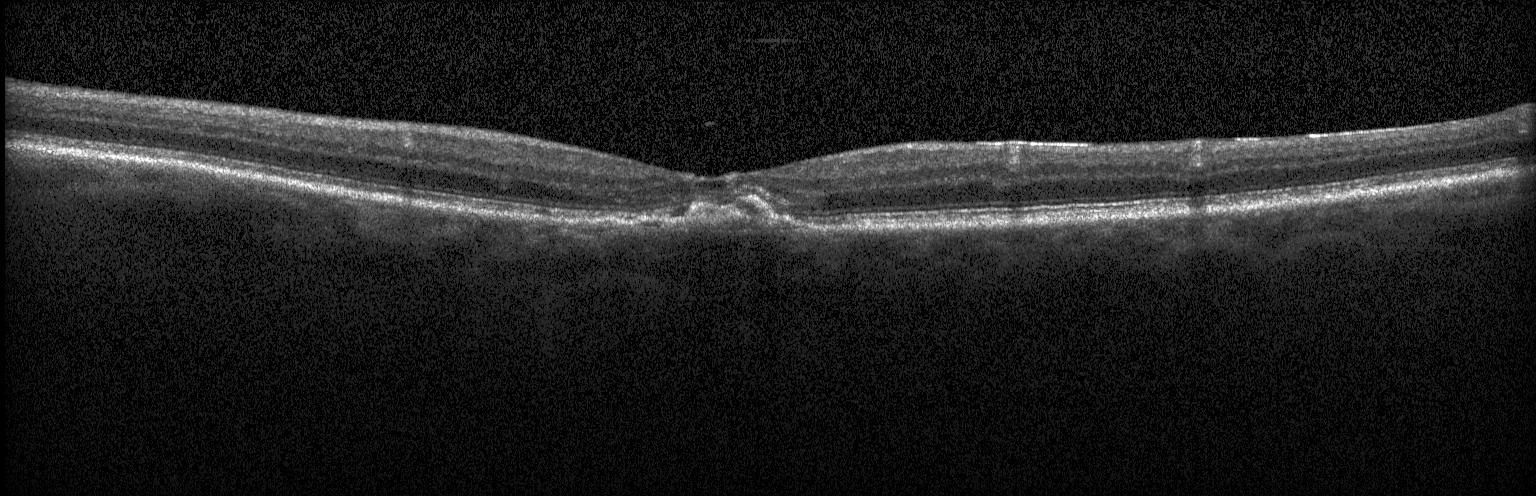

Acquired on a Heidelberg Spectralis. SD-OCT. Retinal OCT B-scan. Impression: a choroidal neovascular membrane.